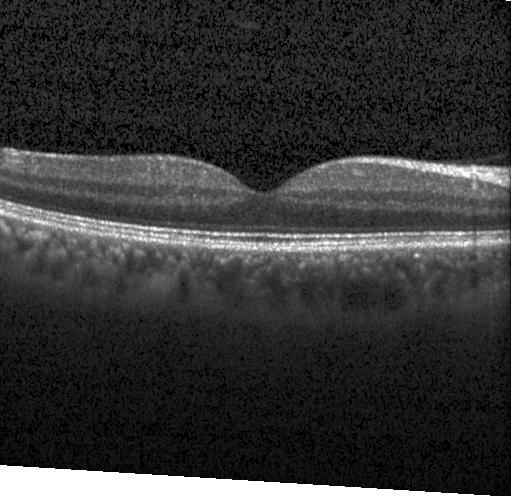 Retinal OCT cross-section.
Assessment: neither CNV, DME, nor drusen.